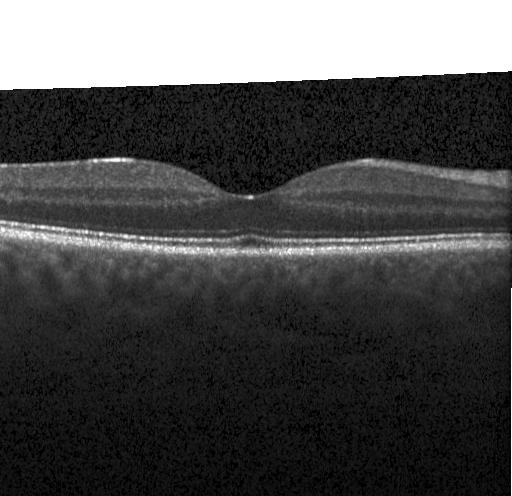 Heidelberg Spectralis OCT system; optical coherence tomography scan; SD-OCT. The scan shows no CNV, DME, or drusen.